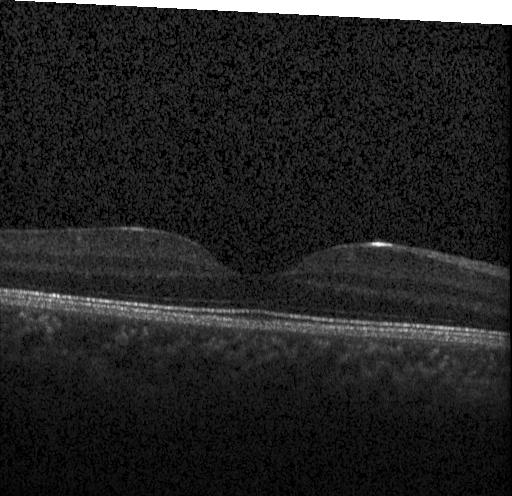 Centered on the fovea, spectral-domain optical coherence tomography, retinal OCT B-scan, Heidelberg Spectralis.
Impression: no choroidal neovascularization, no diabetic macular edema, and no drusen.